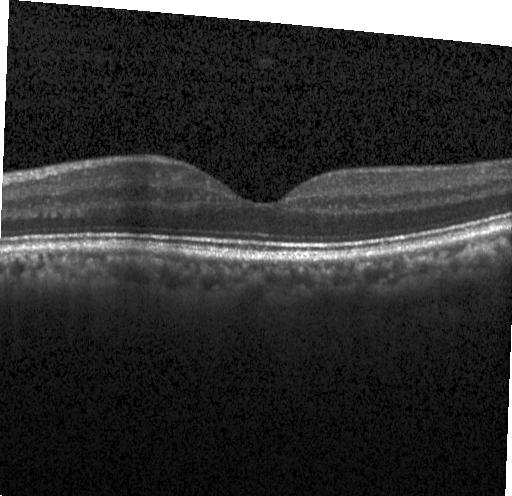 Retinal OCT cross-section.
Assessment: no choroidal neovascularization, diabetic macular edema, or drusen.